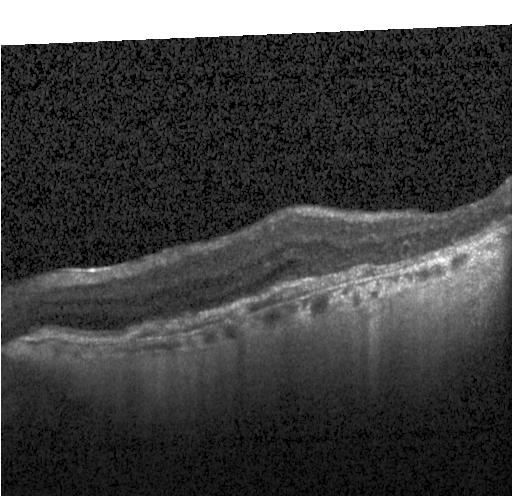
Fovea-centered · OCT line scan · Heidelberg Spectralis OCT system · SD-OCT. Finding: a choroidal neovascular membrane.